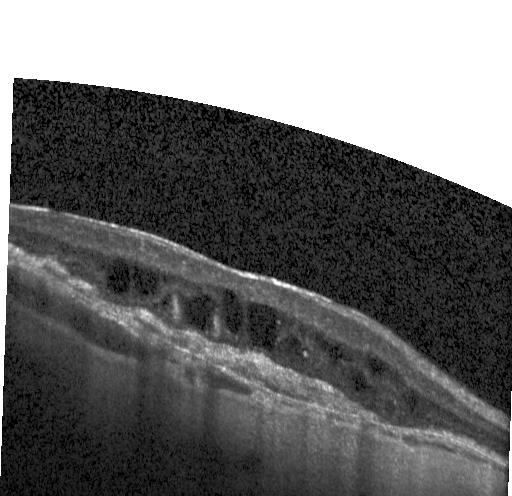 Finding: choroidal neovascularization.